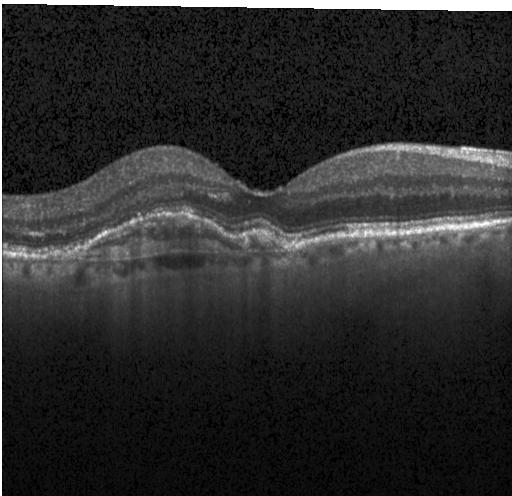

Spectral-domain optical coherence tomography · instrument: Heidelberg Spectralis · optical coherence tomography B-scan
Impression: choroidal neovascularization (CNV).